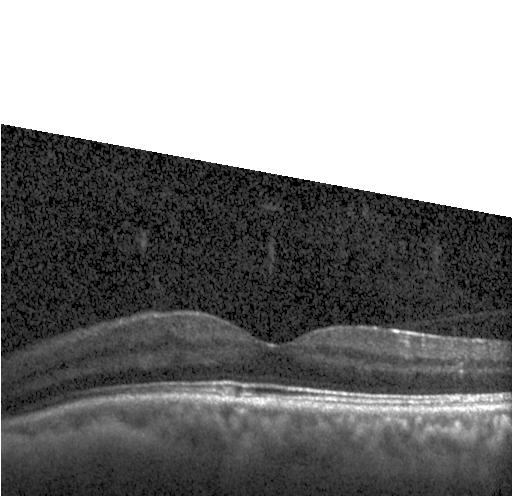 OCT line scan; acquired on a Heidelberg Spectralis; centered on the fovea. OCT finding: neither choroidal neovascularization, diabetic macular edema, nor drusen.